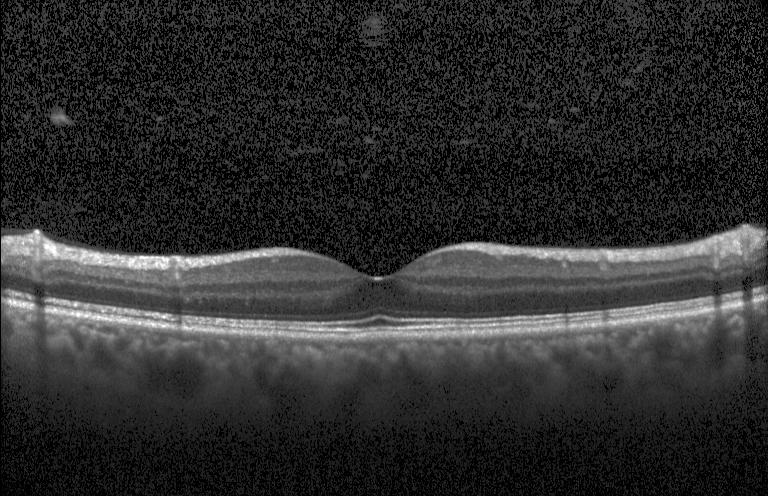 OCT line scan
Assessment: no evidence of choroidal neovascularization, diabetic macular edema, or drusen.